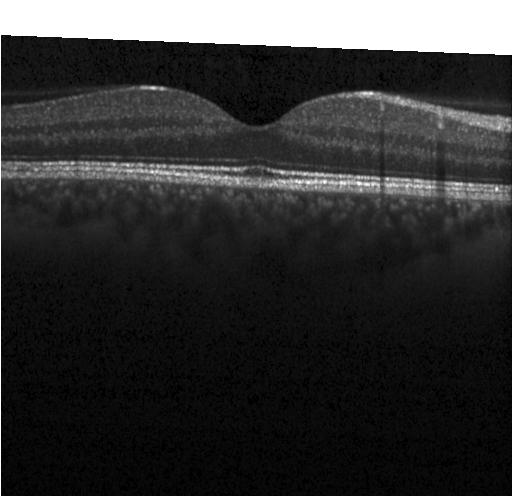 Dx: no CNV, DME, or drusen.